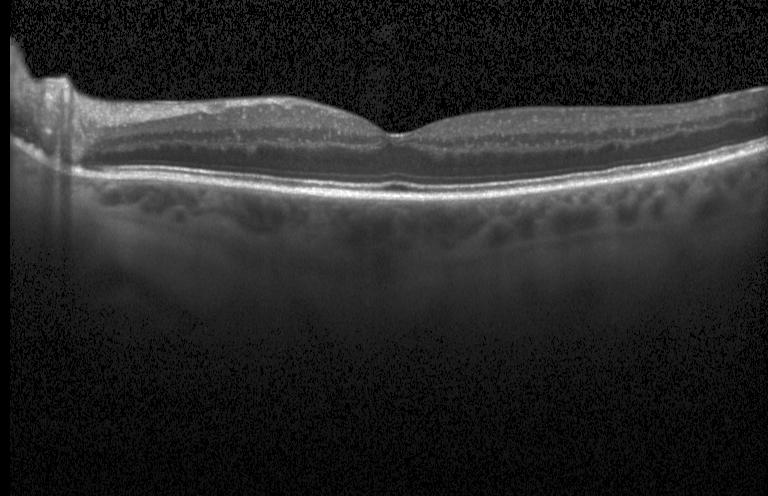
Retinal OCT B-scan. Instrument: Heidelberg Spectralis
No CNV, DME, or drusen.